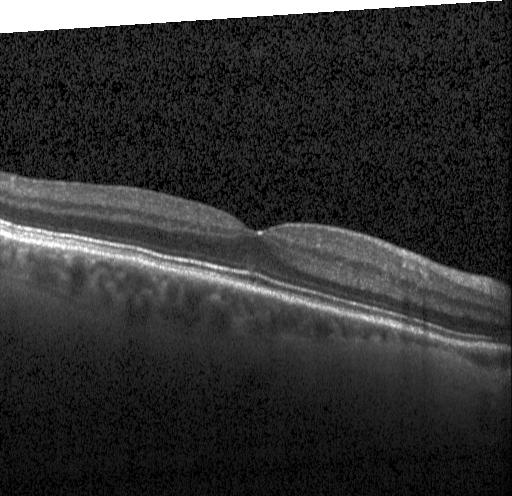 Spectral-domain optical coherence tomography; optical coherence tomography B-scan; horizontal scan through the fovea — Diagnosis: neither CNV, DME, nor drusen.